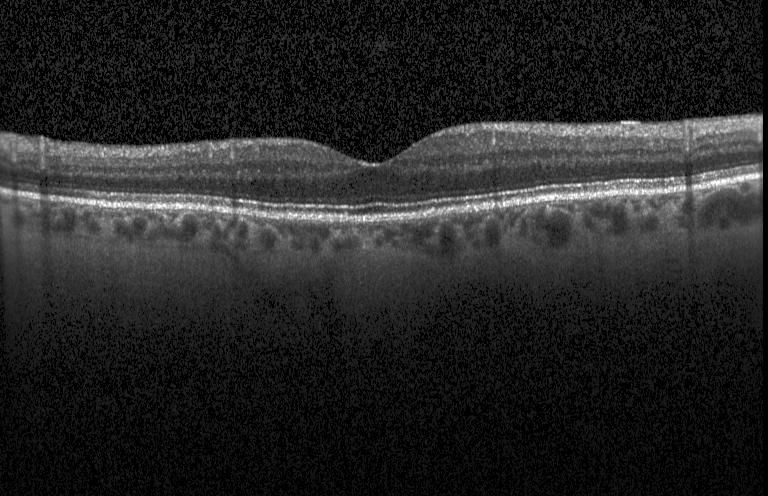
OCT scan showing no choroidal neovascularization, diabetic macular edema, or drusen.